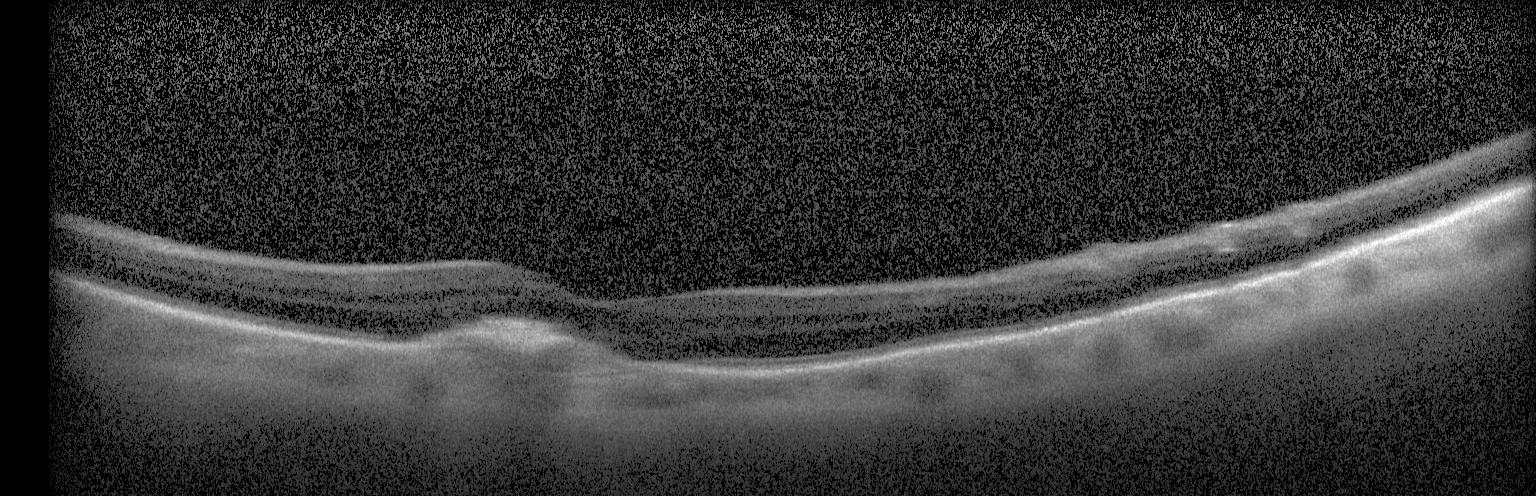
Impression: a choroidal neovascular membrane.